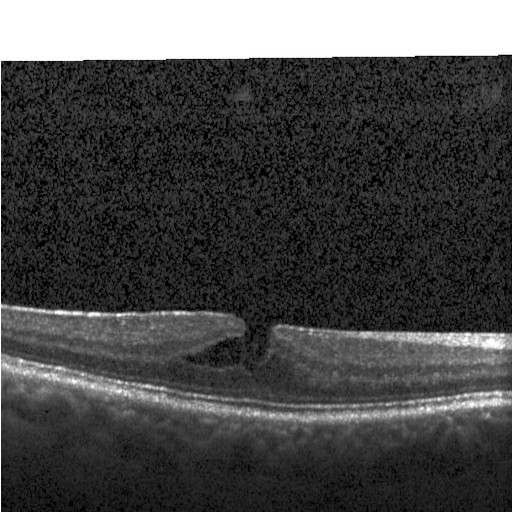
Macular OCT: DME.